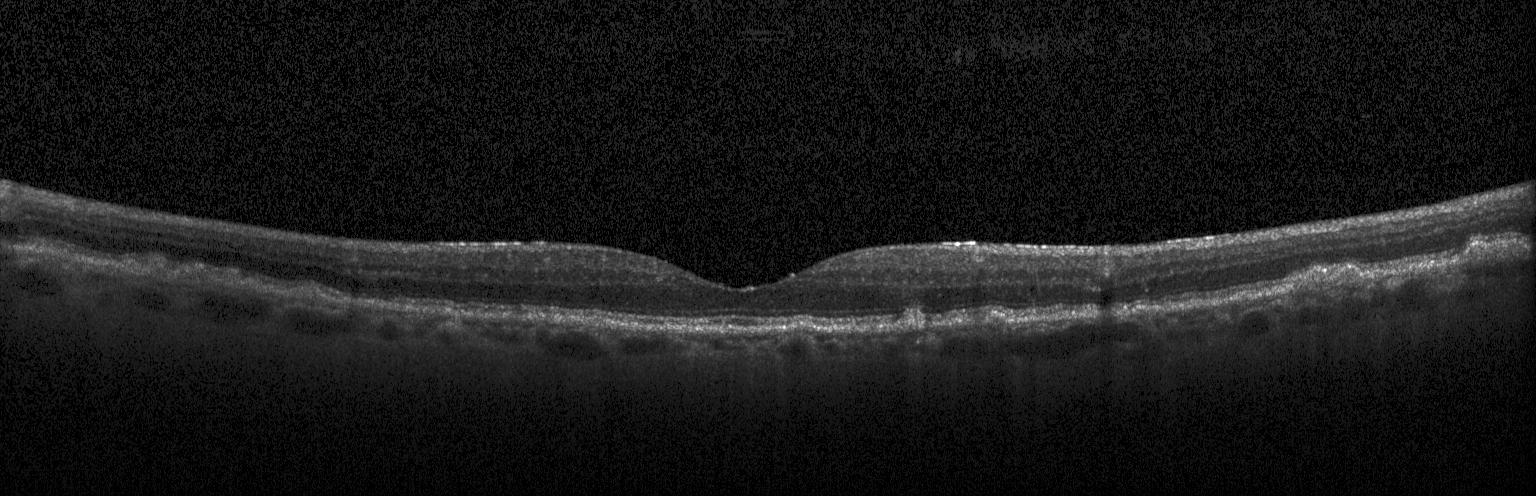

OCT B-scan.
Assessment: multiple drusen.